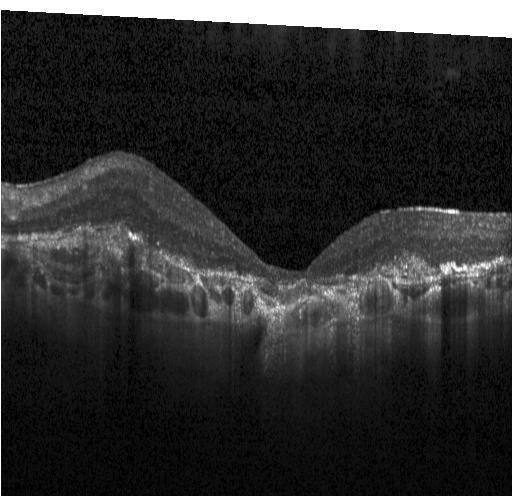
Retinal OCT cross-section · centered on the fovea — Impression: a choroidal neovascular membrane.